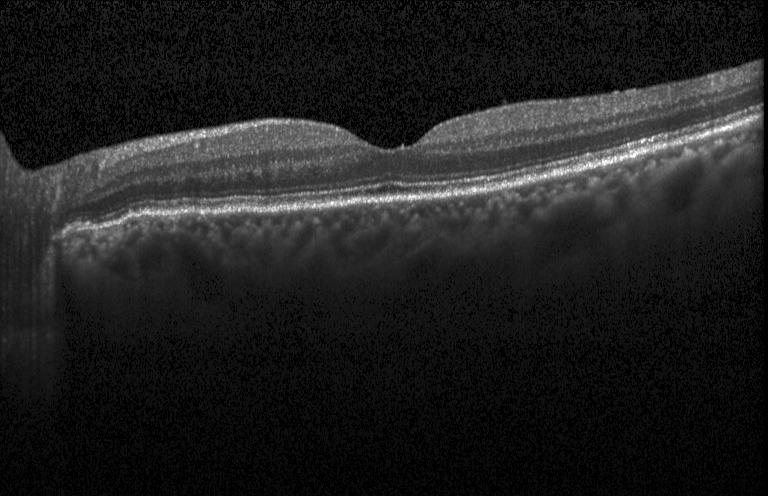
Spectral-domain optical coherence tomography; acquired on a Heidelberg Spectralis; optical coherence tomography B-scan — This B-scan demonstrates neither choroidal neovascularization, diabetic macular edema, nor drusen.